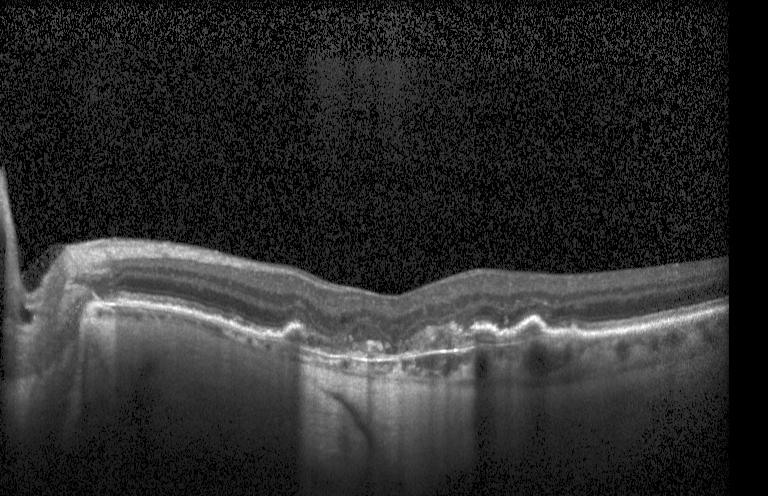 Diagnosis: choroidal neovascularization.